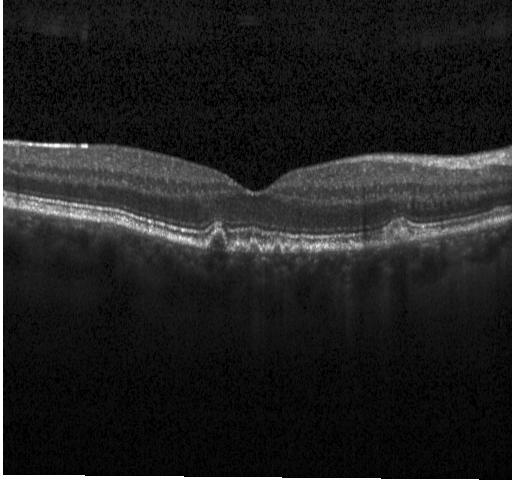
Horizontal scan through the fovea, retinal OCT B-scan, instrument: Heidelberg Spectralis.
Finding: multiple drusen.